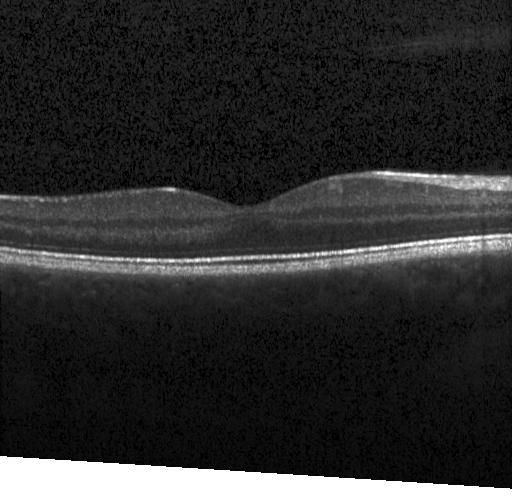

Macular OCT: no choroidal neovascularization, diabetic macular edema, or drusen.